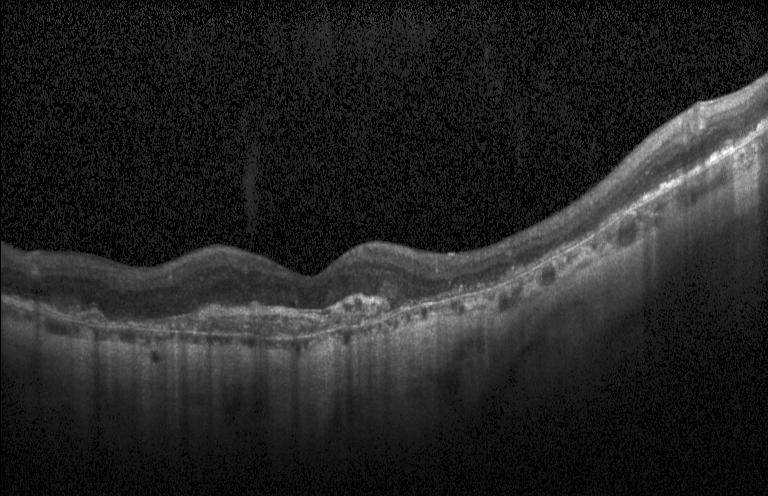
Fovea-centered, Heidelberg Spectralis OCT system, SD-OCT, OCT B-scan.
Diagnosis: choroidal neovascularization (CNV).